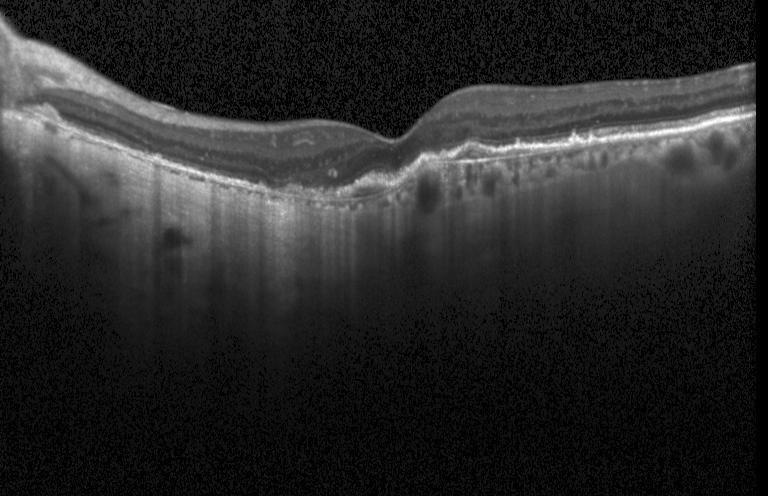 OCT B-scan showing a choroidal neovascular membrane.